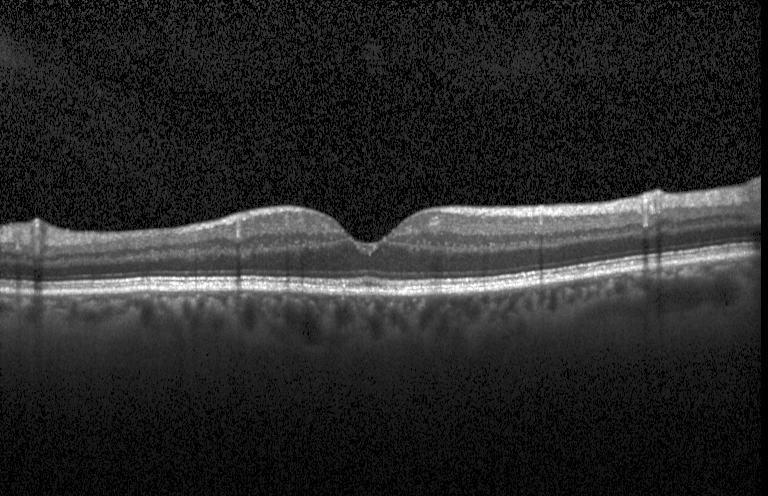 Heidelberg Spectralis OCT system · optical coherence tomography scan — Impression: no choroidal neovascularization, diabetic macular edema, or drusen.